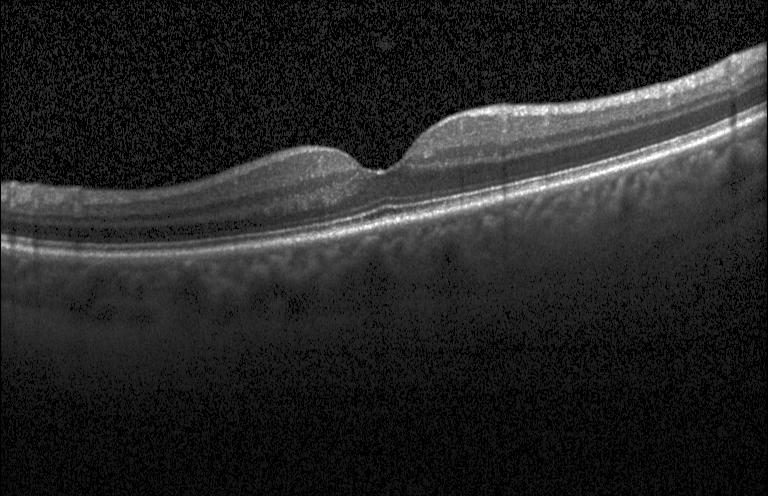

Diagnosis: no evidence of CNV, DME, or drusen.